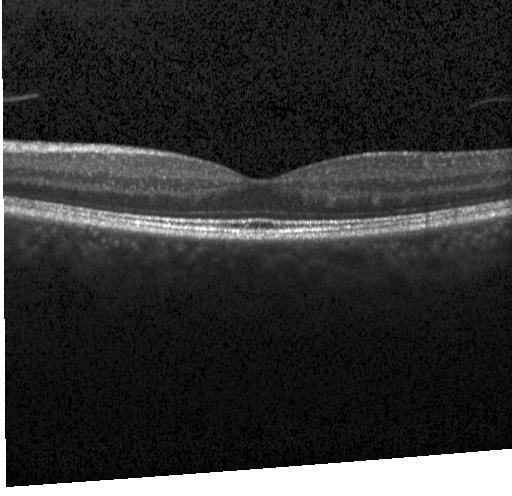

Fovea-centered, Heidelberg Spectralis OCT system, retinal OCT cross-section
Diagnosis: neither choroidal neovascularization, diabetic macular edema, nor drusen.